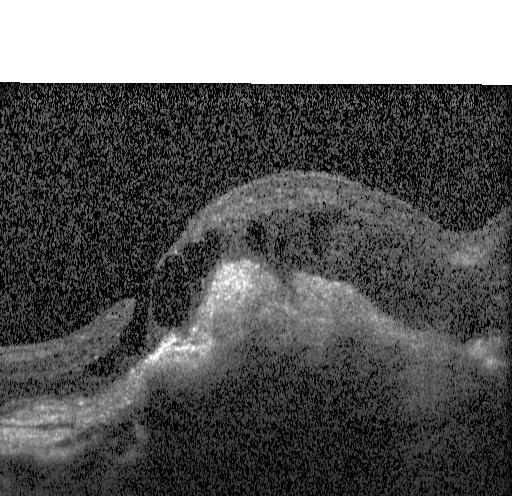

Finding: choroidal neovascularization.